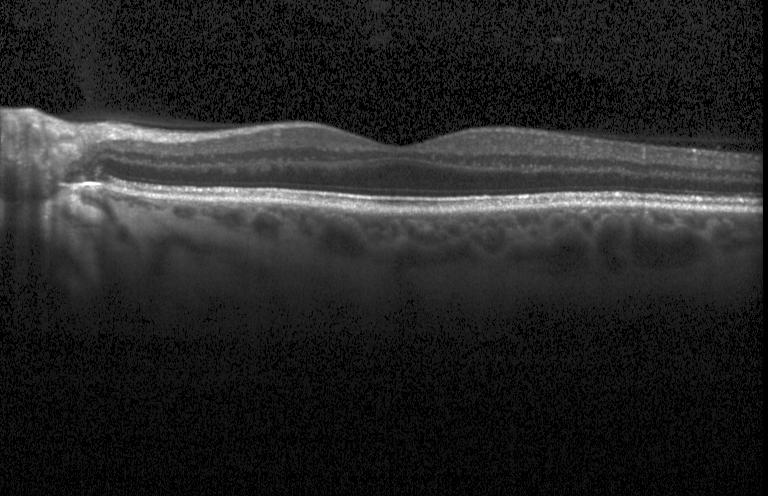 Instrument: Heidelberg Spectralis · OCT B-scan — The scan shows neither choroidal neovascularization, diabetic macular edema, nor drusen.